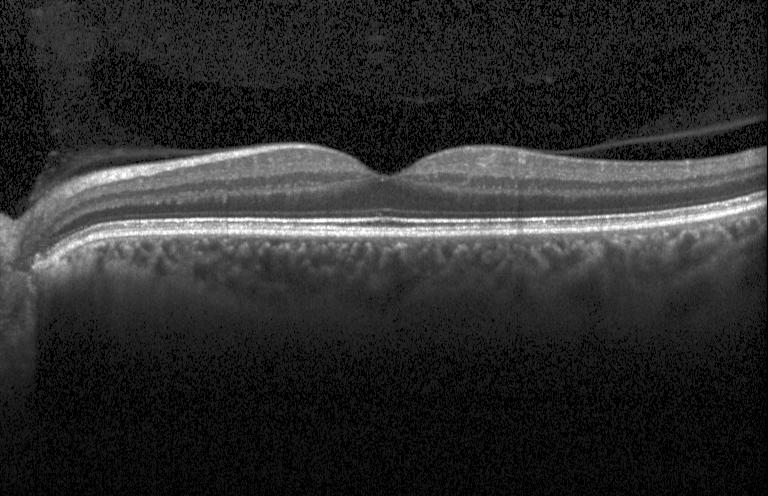

Centered on the fovea. Spectral-domain optical coherence tomography. Retinal OCT B-scan.
Diagnosis: no evidence of CNV, DME, or drusen.